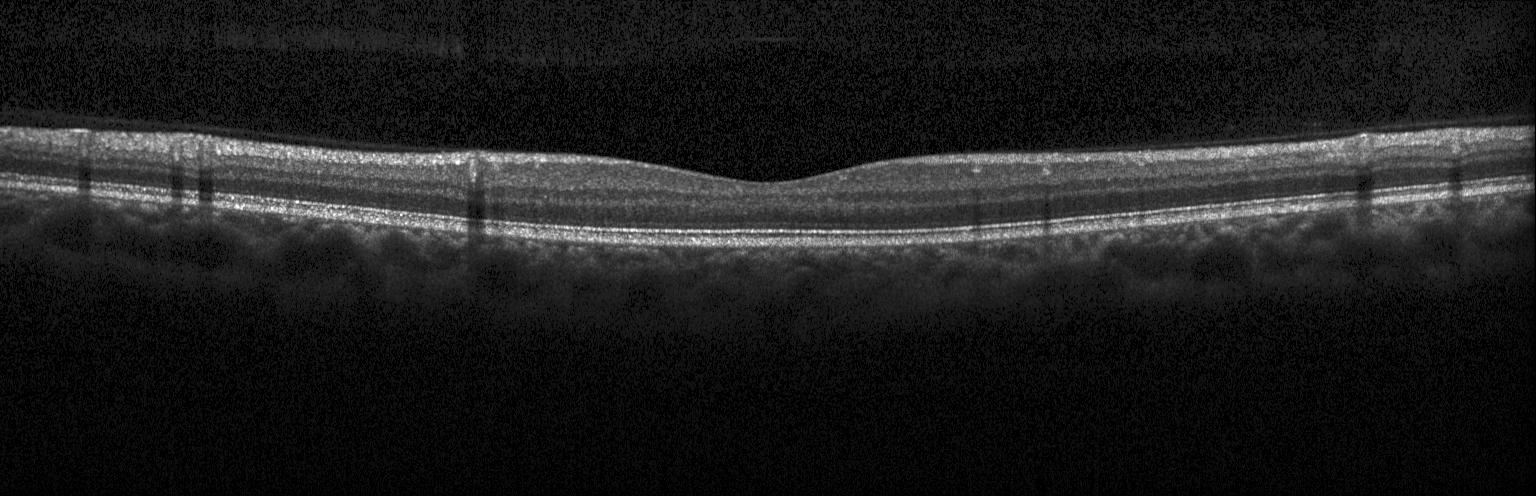

Impression: no evidence of choroidal neovascularization, diabetic macular edema, or drusen.